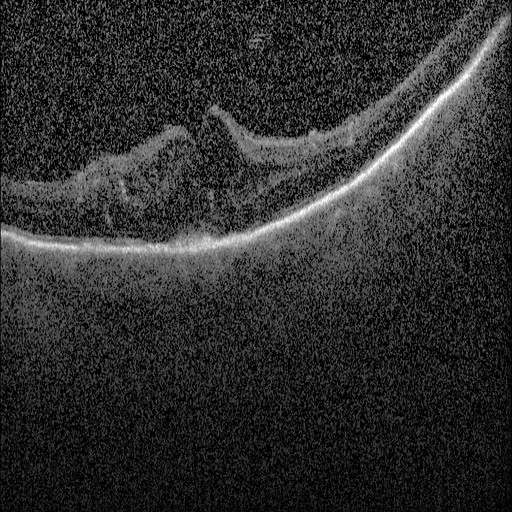
OCT line scan — Diagnosis: diabetic macular edema (DME).